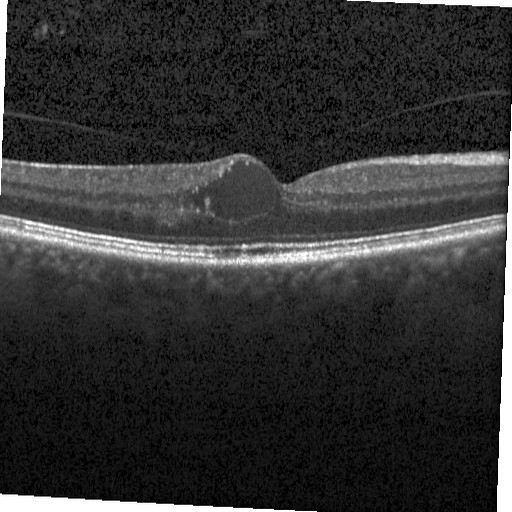 Impression: DME.